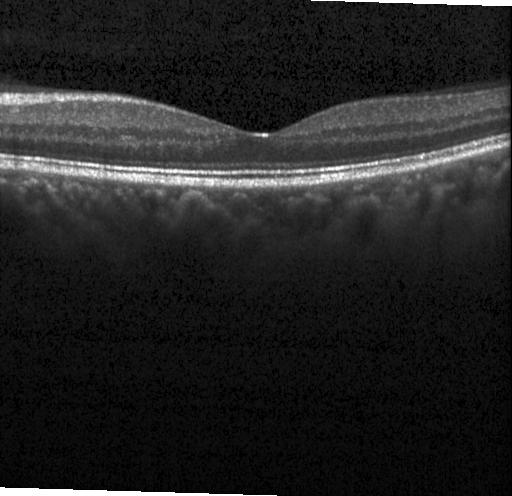

OCT B-scan — This B-scan demonstrates neither choroidal neovascularization, diabetic macular edema, nor drusen.